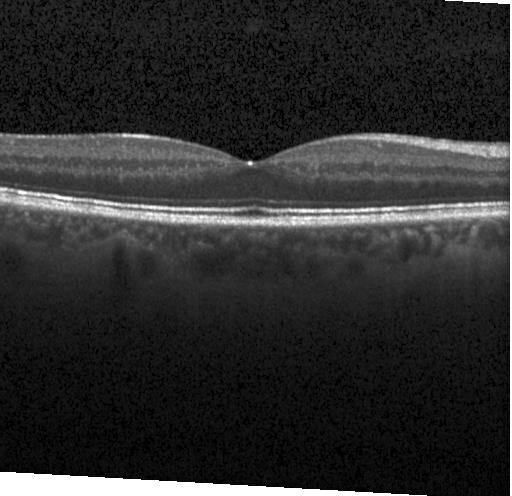
OCT scan showing no choroidal neovascularization, diabetic macular edema, or drusen.